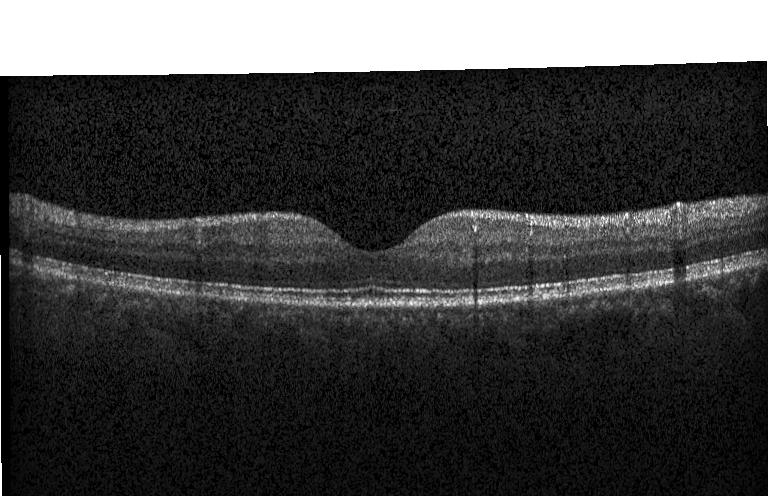

Retinal OCT B-scan, through the macula.
Finding: no choroidal neovascularization, diabetic macular edema, or drusen.